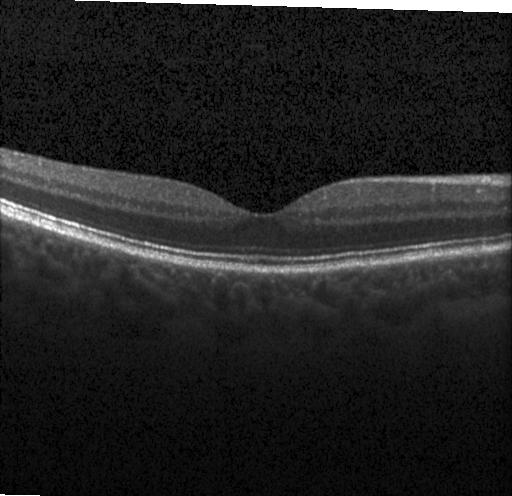
OCT B-scan.
This B-scan demonstrates no evidence of CNV, DME, or drusen.